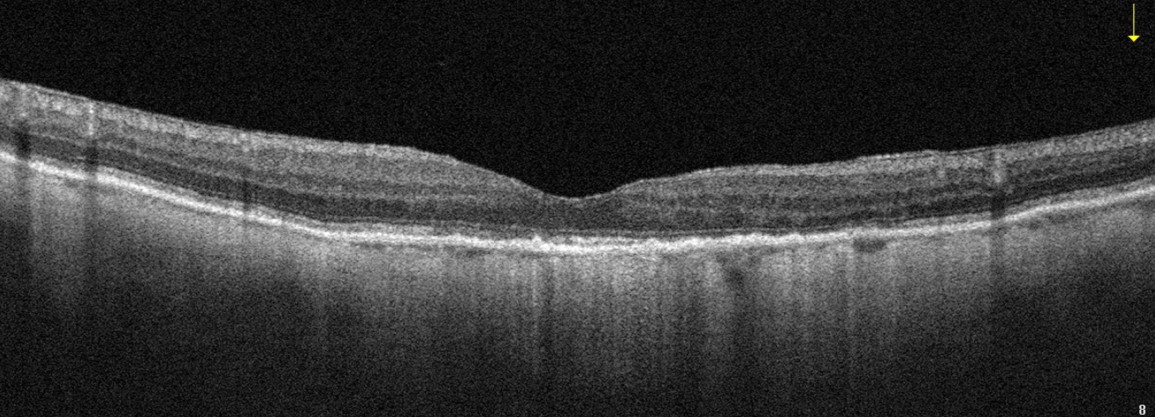
OCT B-scan — This B-scan demonstrates age-related macular degeneration (AMD).